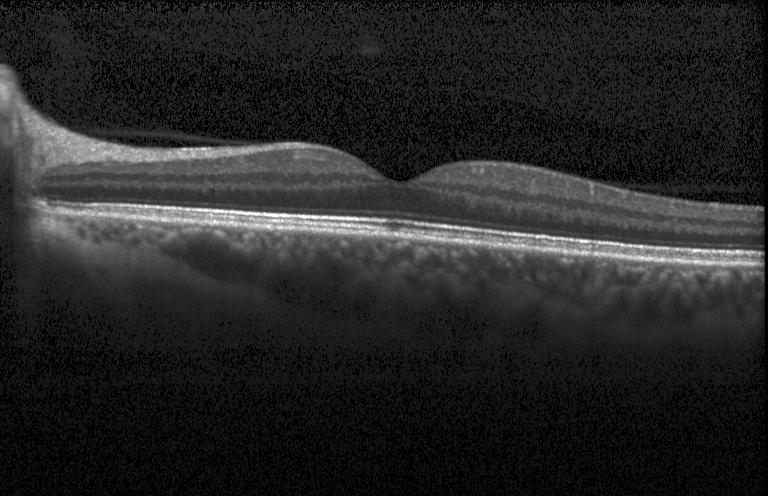

OCT B-scan — Diagnosis: neither CNV, DME, nor drusen.